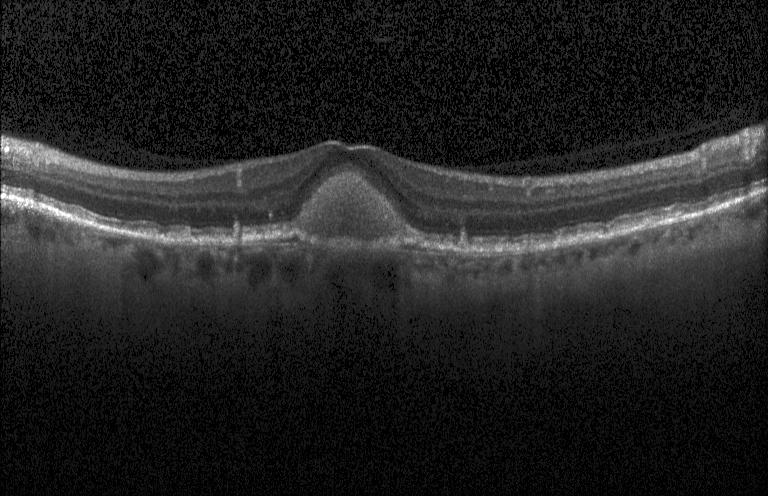 Retinal OCT cross-section.
Impression: a choroidal neovascular membrane.